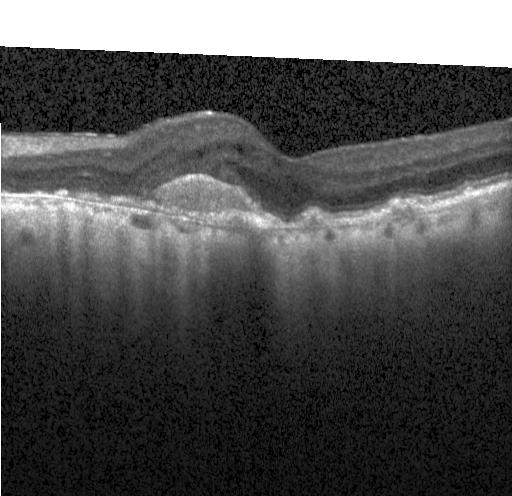 Centered on the fovea. OCT line scan. Instrument: Heidelberg Spectralis. Impression: a choroidal neovascular membrane.